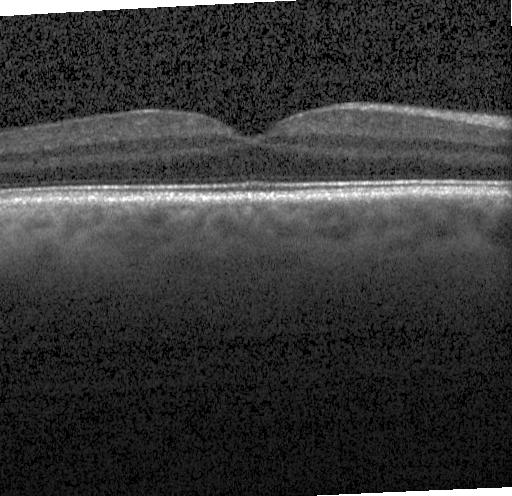
SD-OCT; horizontal scan through the fovea; OCT line scan; instrument: Heidelberg Spectralis. This B-scan demonstrates no evidence of choroidal neovascularization, diabetic macular edema, or drusen.